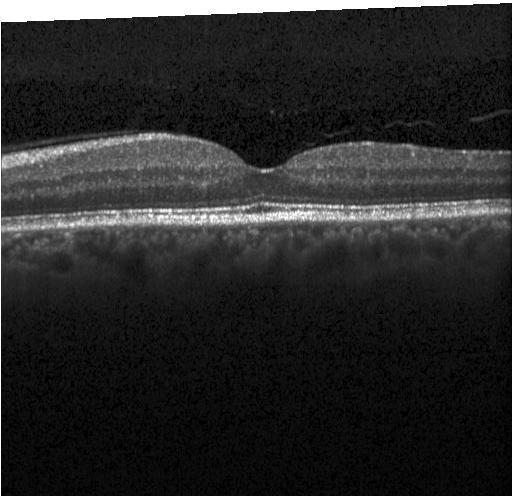
Finding: no choroidal neovascularization, no diabetic macular edema, and no drusen.